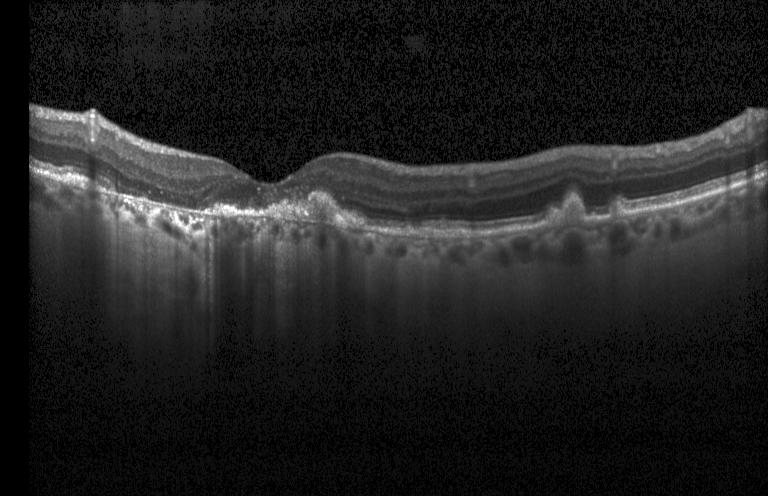 Optical coherence tomography scan.
CNV.